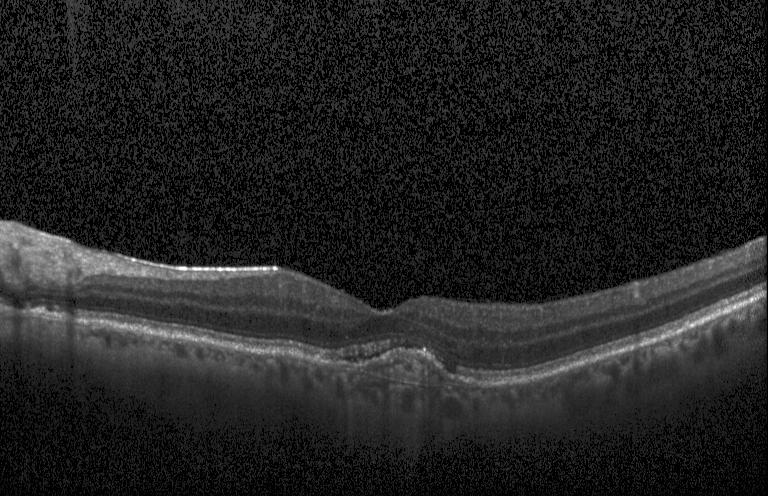 OCT line scan
Macular OCT: a choroidal neovascular membrane.